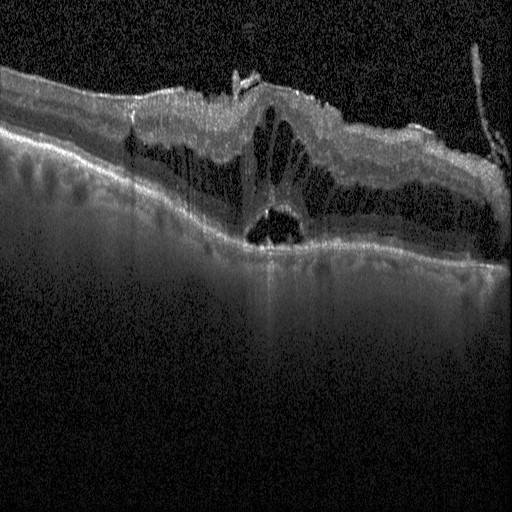

Spectral-domain OCT · retinal OCT B-scan · Heidelberg Spectralis
Assessment: DME.